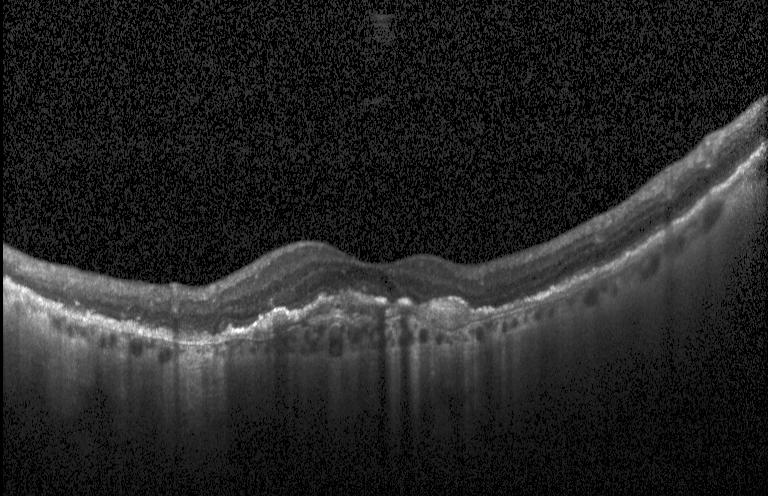

OCT finding: a choroidal neovascular membrane.